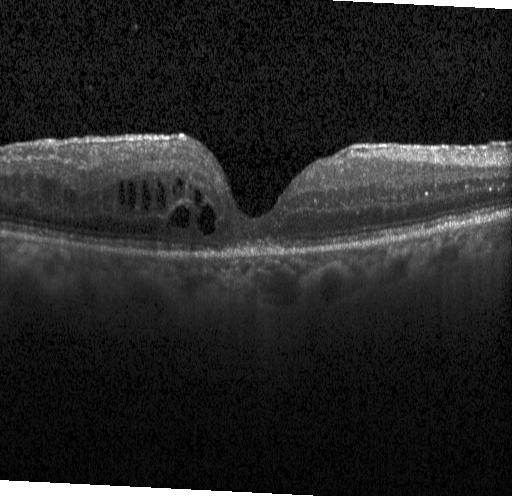 OCT finding: DME.